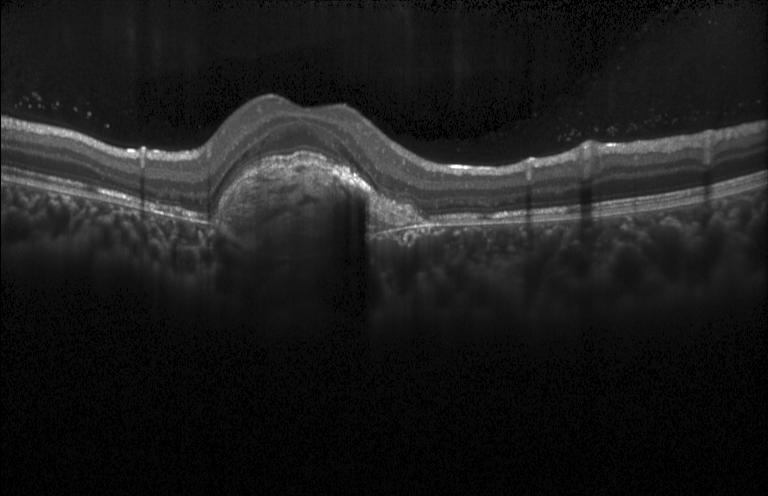
The scan shows CNV.